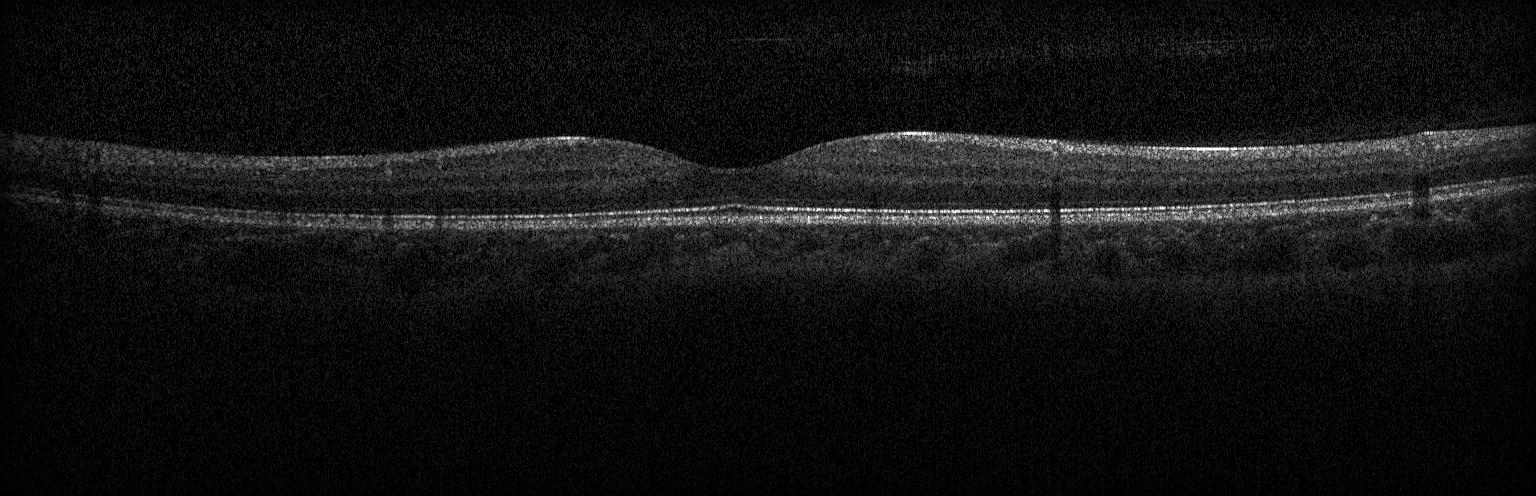

Optical coherence tomography scan — Diagnosis: no choroidal neovascularization, no diabetic macular edema, and no drusen.